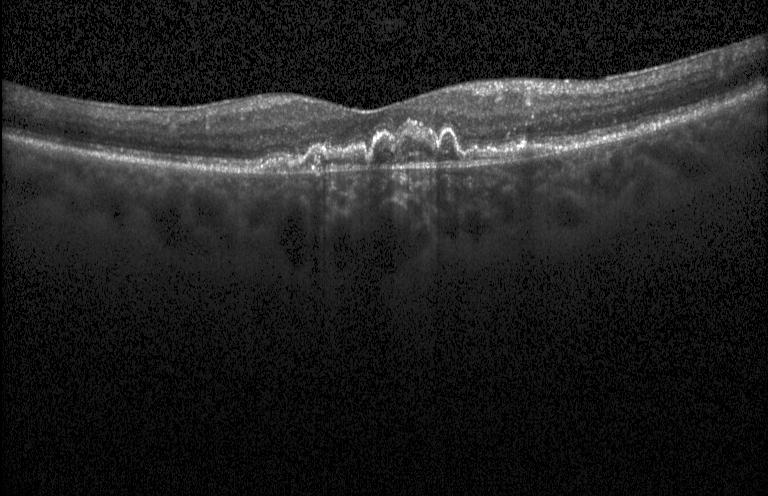
Retinal OCT cross-section showing CNV.